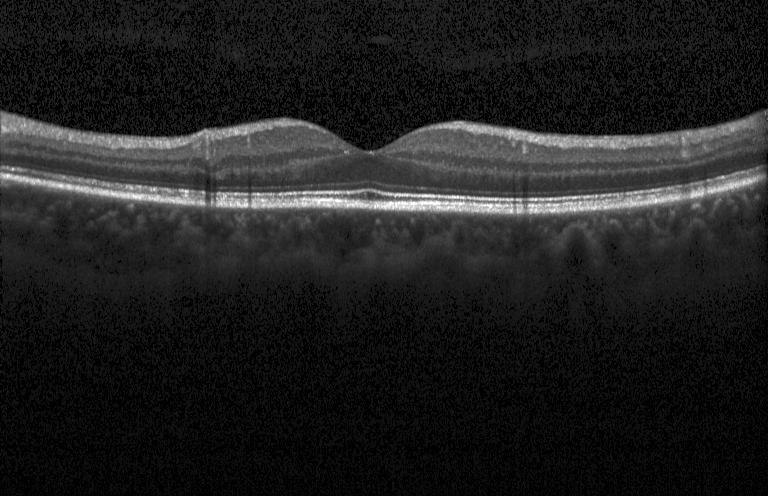
Macular scan · optical coherence tomography scan · Heidelberg Spectralis OCT system · spectral-domain OCT
The scan shows no evidence of choroidal neovascularization, diabetic macular edema, or drusen.